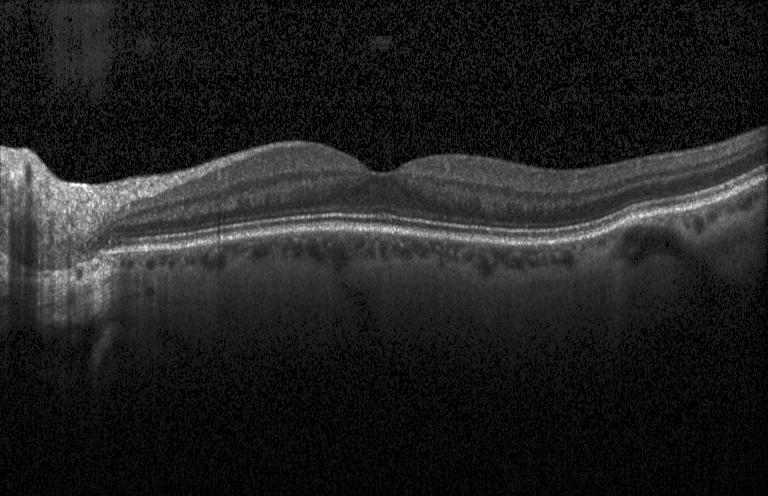

Spectral-domain OCT · macular scan · Heidelberg Spectralis OCT system · optical coherence tomography scan — Diagnosis: no evidence of choroidal neovascularization, diabetic macular edema, or drusen.